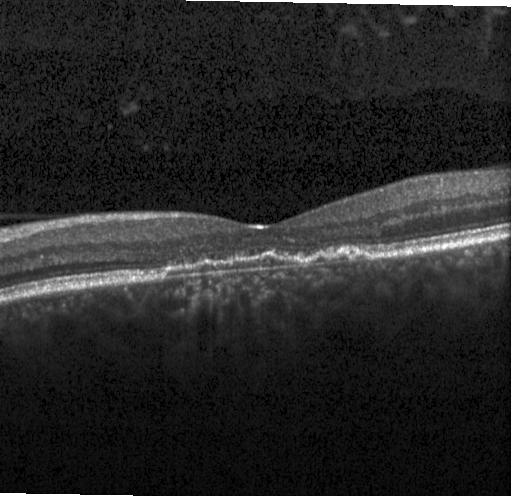

Horizontal scan through the fovea. OCT line scan. Acquired on a Heidelberg Spectralis
Finding: a choroidal neovascular membrane.